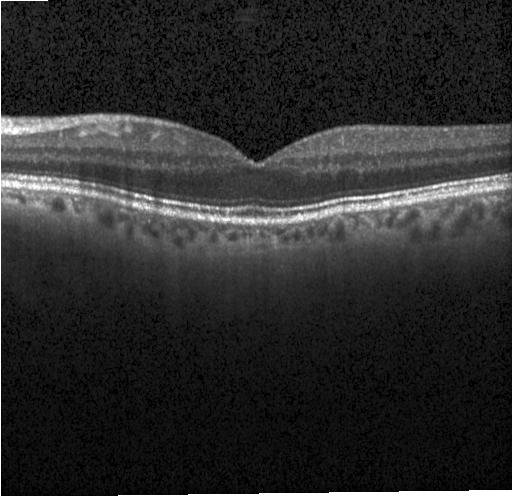
Heidelberg Spectralis. Retinal OCT B-scan. Spectral-domain OCT. Horizontal scan through the fovea. This B-scan demonstrates no evidence of choroidal neovascularization, diabetic macular edema, or drusen.